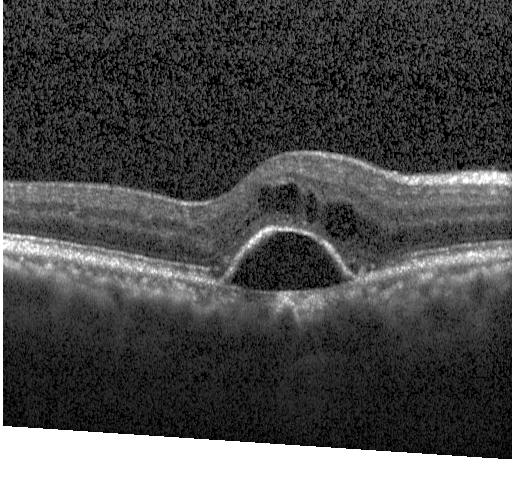 Retinal OCT B-scan — OCT finding: a choroidal neovascular membrane.